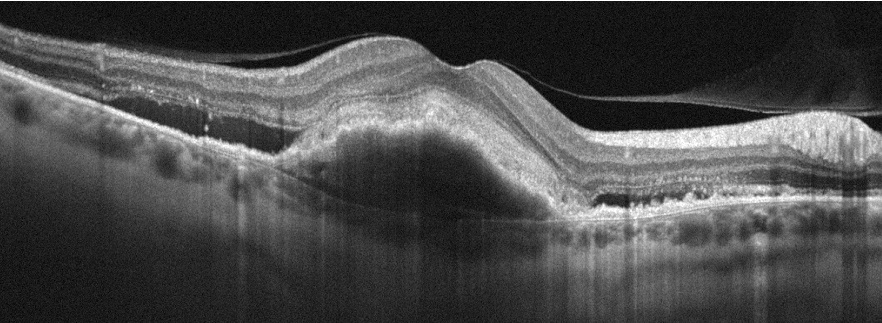

Fovea-centered; instrument: Optovue Avanti RTVue XR; optical coherence tomography B-scan. This B-scan demonstrates AMD.